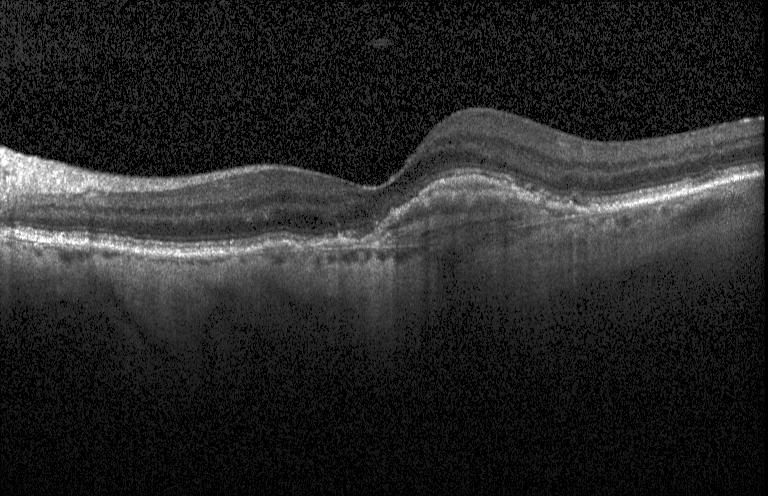

Spectral-domain OCT. OCT line scan. Heidelberg Spectralis OCT system — Impression: a choroidal neovascular membrane.